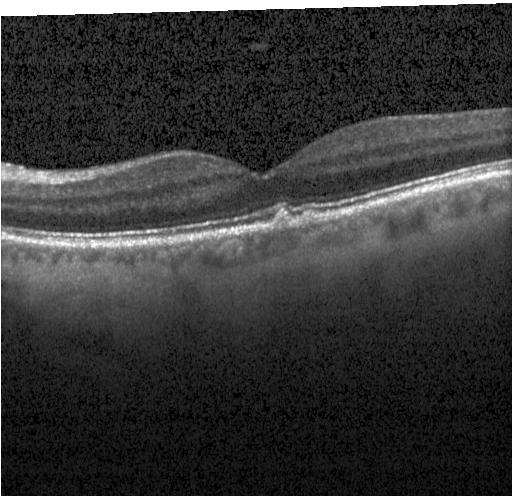

Spectral-domain OCT B-scan: drusen.